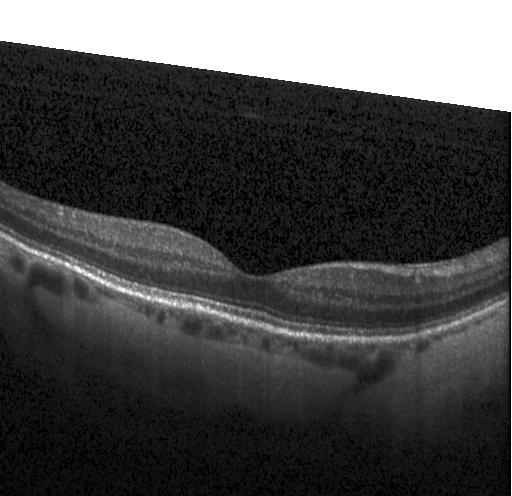 Optical coherence tomography scan. No choroidal neovascularization, diabetic macular edema, or drusen.